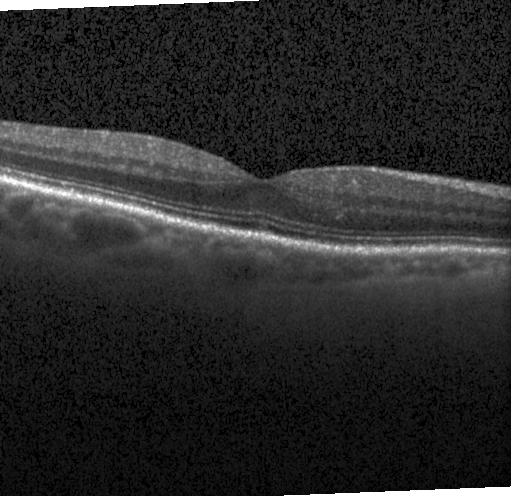 Optical coherence tomography B-scan · Heidelberg Spectralis OCT system. Diagnosis: no evidence of choroidal neovascularization, diabetic macular edema, or drusen.